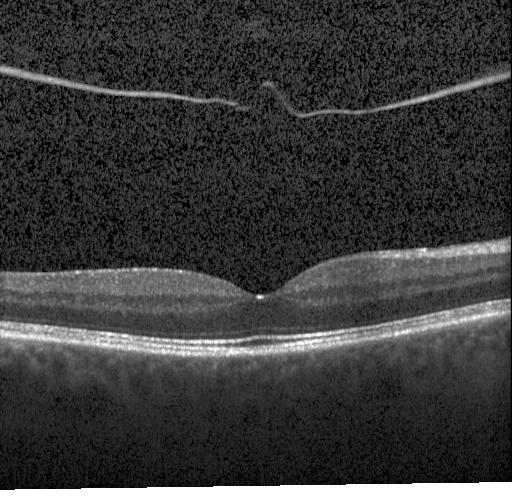
Retinal OCT cross-section showing neither choroidal neovascularization, diabetic macular edema, nor drusen.